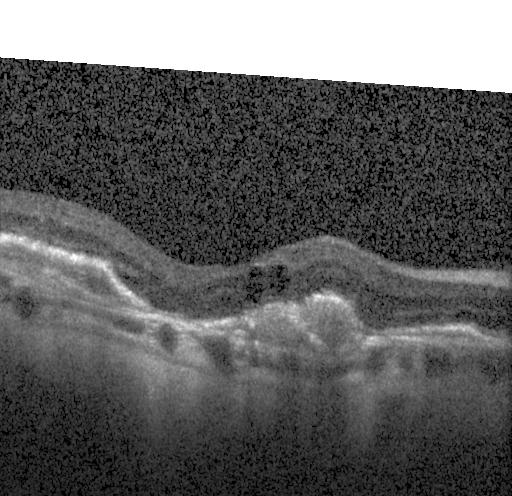 Macular OCT demonstrating CNV.